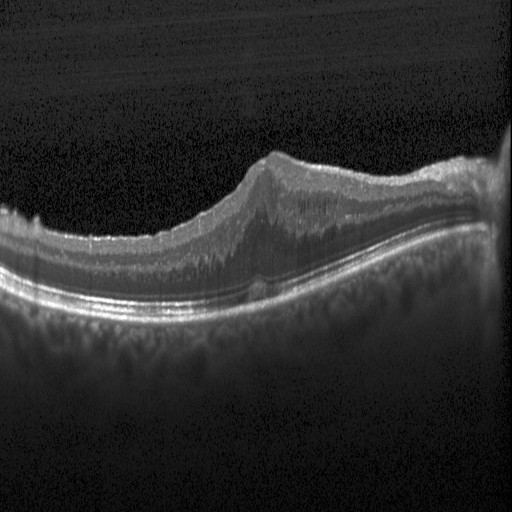
Centered on the fovea. SD-OCT. Retinal OCT cross-section.
Diagnosis: DME.